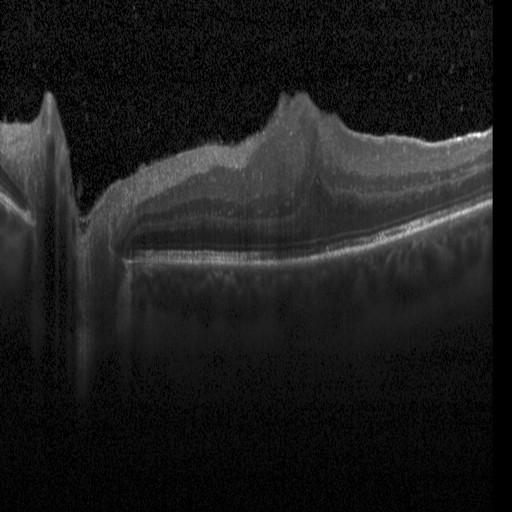
Instrument: Heidelberg Spectralis; spectral-domain OCT; through the macula; optical coherence tomography scan
Finding: diabetic macular edema (DME).